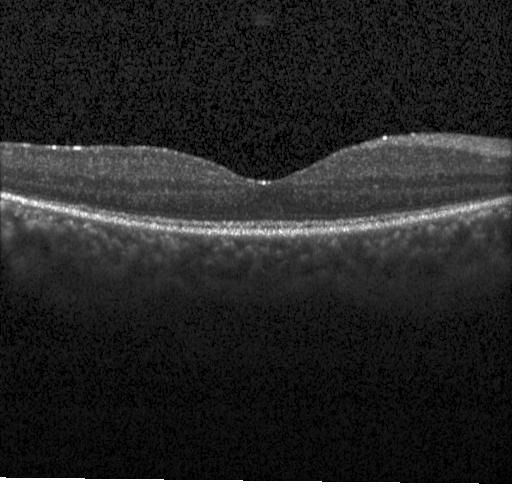

OCT finding: no evidence of choroidal neovascularization, diabetic macular edema, or drusen.